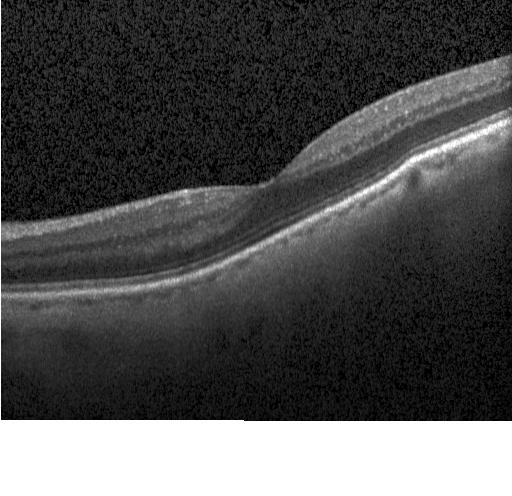 Spectral-domain OCT B-scan: no evidence of choroidal neovascularization, diabetic macular edema, or drusen.